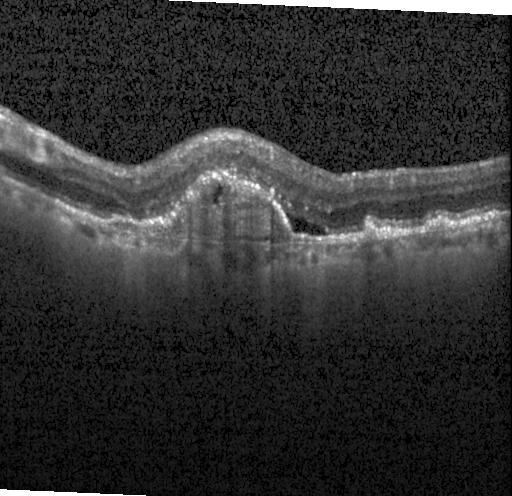

OCT B-scan · instrument: Heidelberg Spectralis — Assessment: choroidal neovascularization (CNV).